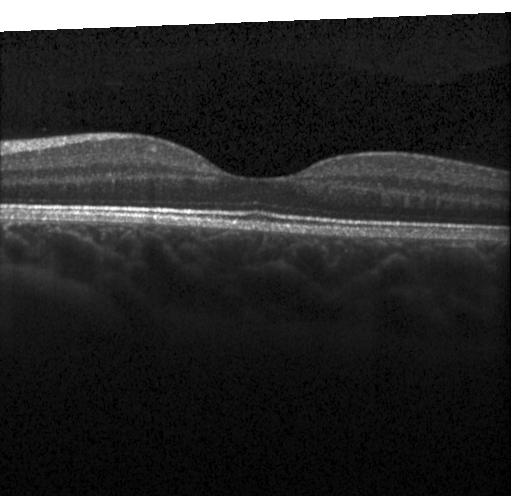
Dx: neither choroidal neovascularization, diabetic macular edema, nor drusen.